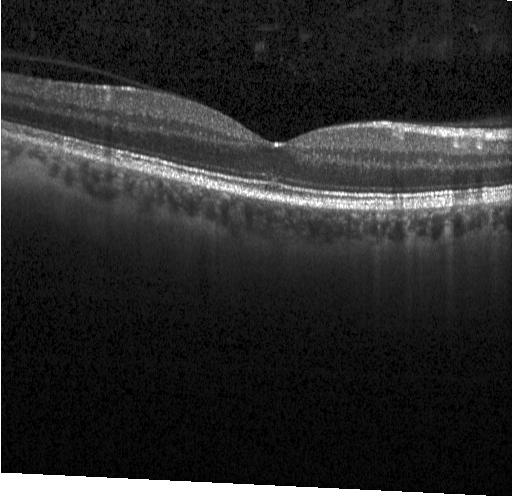 Optical coherence tomography B-scan · spectral-domain optical coherence tomography — OCT finding: no evidence of choroidal neovascularization, diabetic macular edema, or drusen.